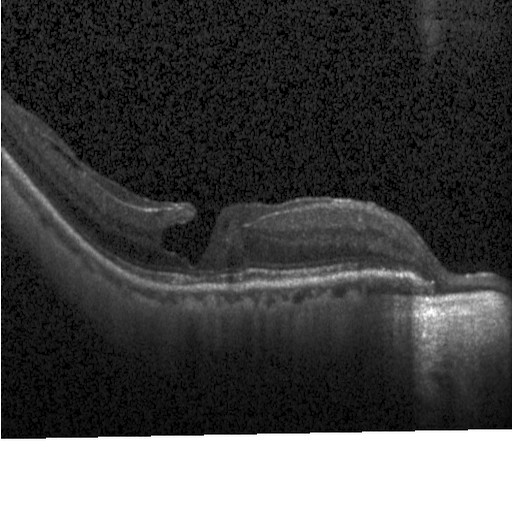 The scan shows diabetic macular edema (DME).